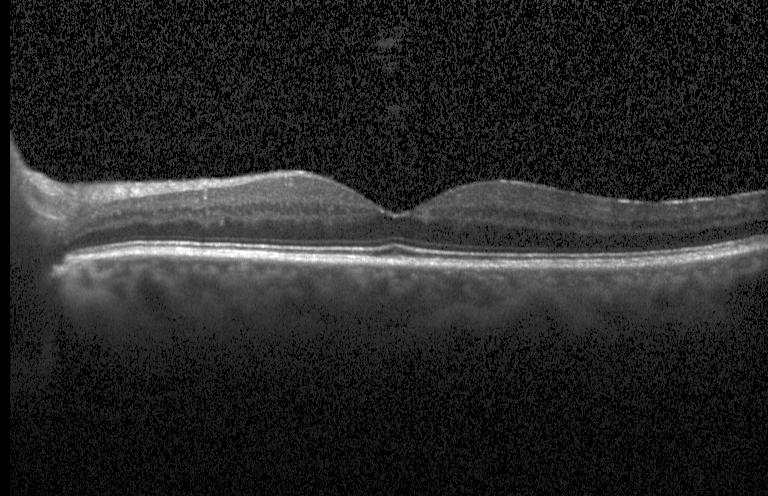

Heidelberg Spectralis, optical coherence tomography B-scan.
Assessment: no choroidal neovascularization, no diabetic macular edema, and no drusen.